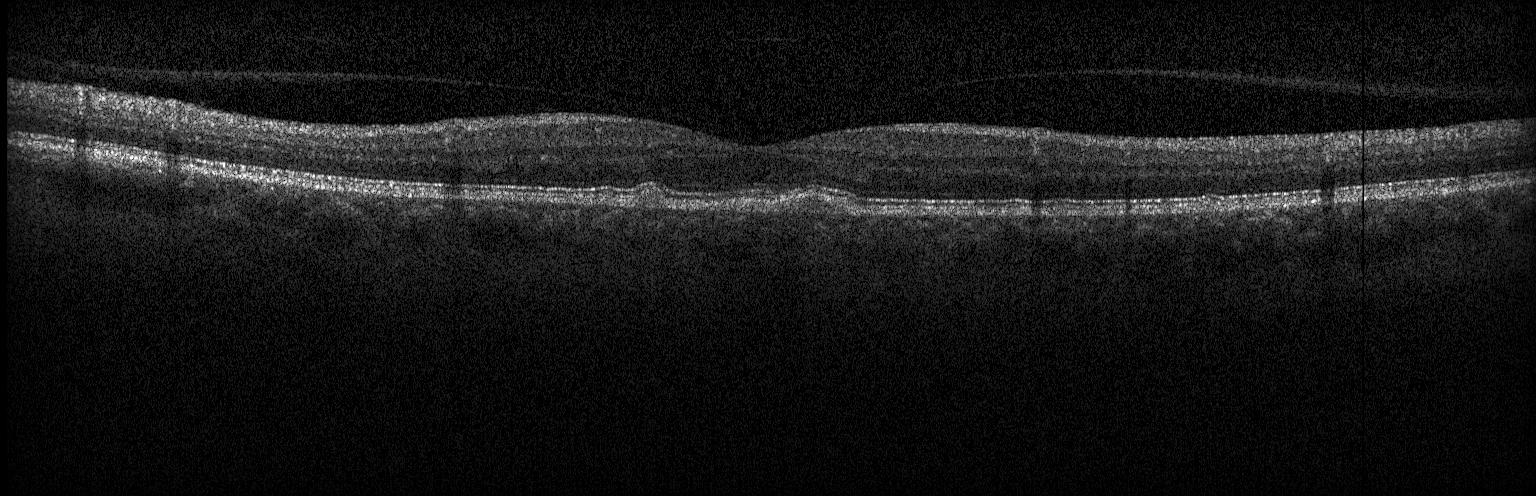
Optical coherence tomography B-scan — Finding: sub-RPE drusenoid deposits.